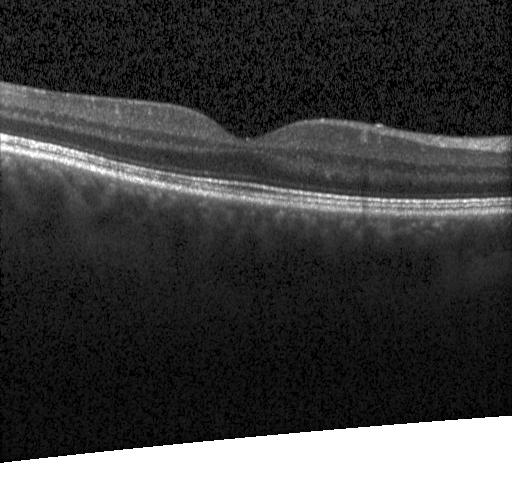
Optical coherence tomography scan · fovea-centered · Heidelberg Spectralis OCT system.
OCT finding: no choroidal neovascularization, diabetic macular edema, or drusen.